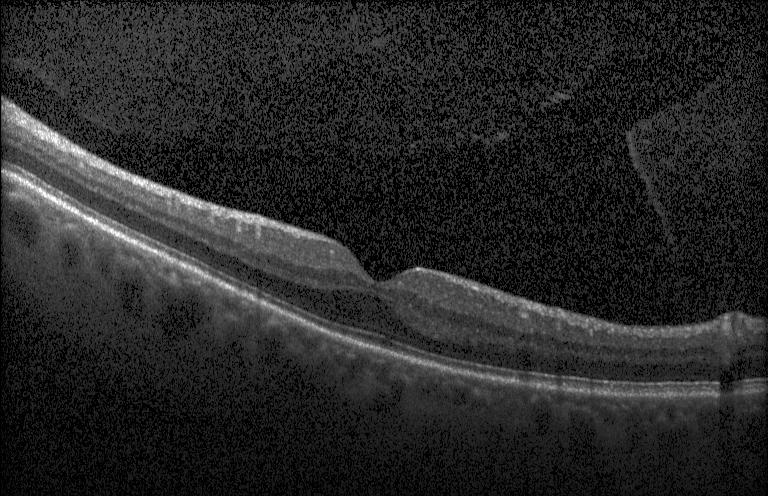 Centered on the fovea; OCT line scan.
Macular OCT: no evidence of CNV, DME, or drusen.